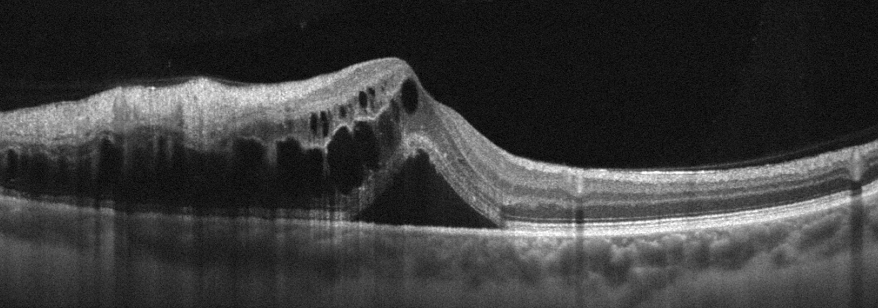
Instrument: Optovue Avanti RTVue XR · OCT line scan
Diagnosis: RVO.